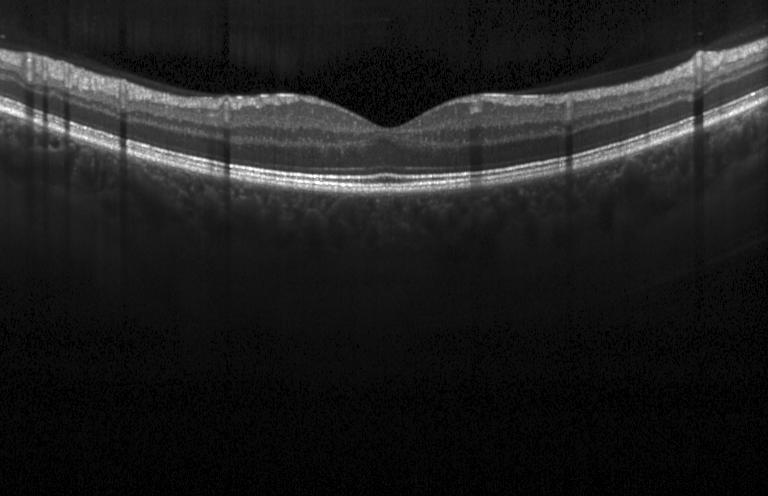
Retinal OCT B-scan
Dx: no choroidal neovascularization, no diabetic macular edema, and no drusen.